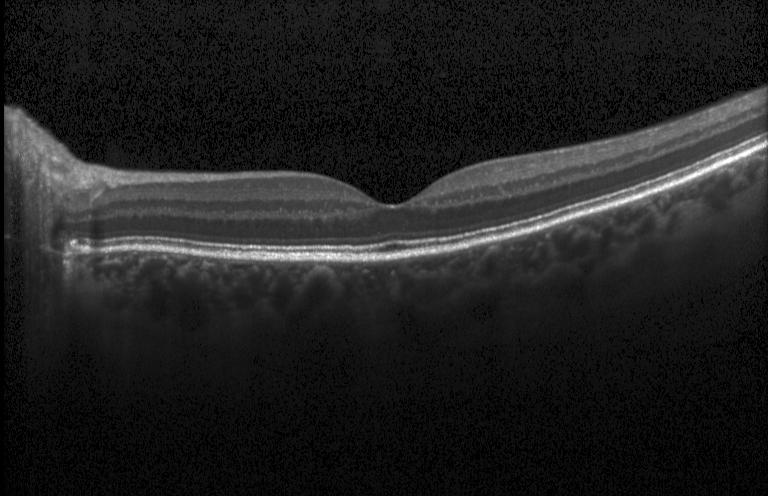
OCT scan showing no choroidal neovascularization, no diabetic macular edema, and no drusen.